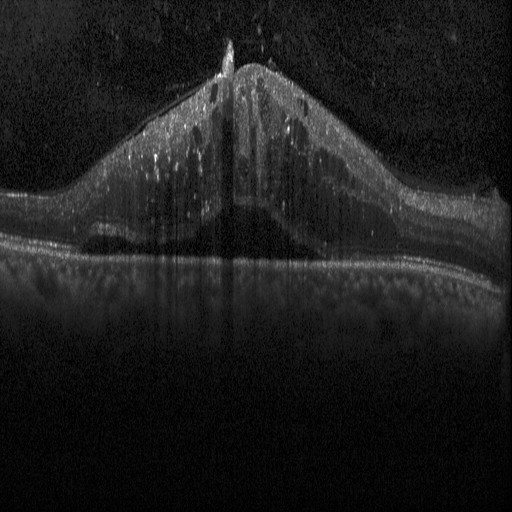 OCT finding: diabetic macular edema (DME).